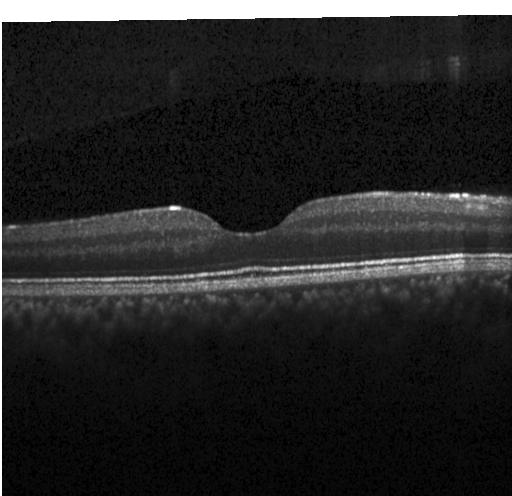
Impression: no choroidal neovascularization, diabetic macular edema, or drusen.